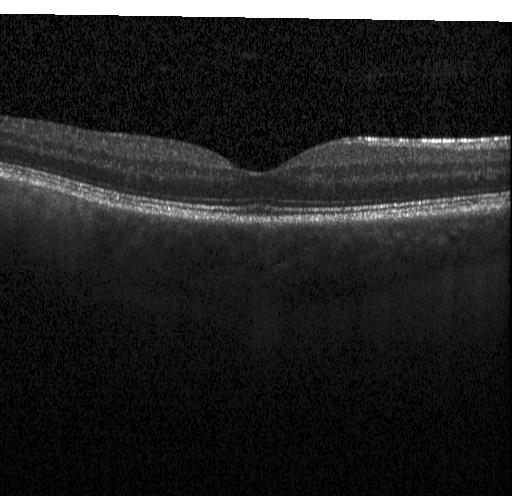 Heidelberg Spectralis. OCT line scan
Impression: no CNV, no DME, and no drusen.